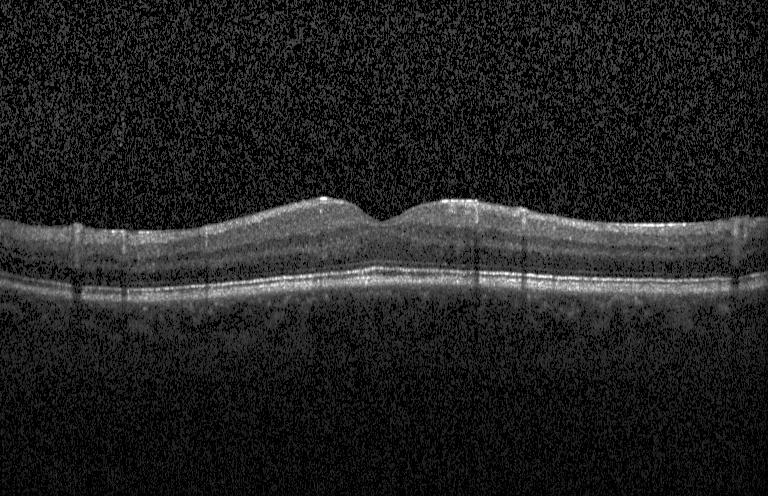

OCT B-scan
Assessment: no choroidal neovascularization, diabetic macular edema, or drusen.